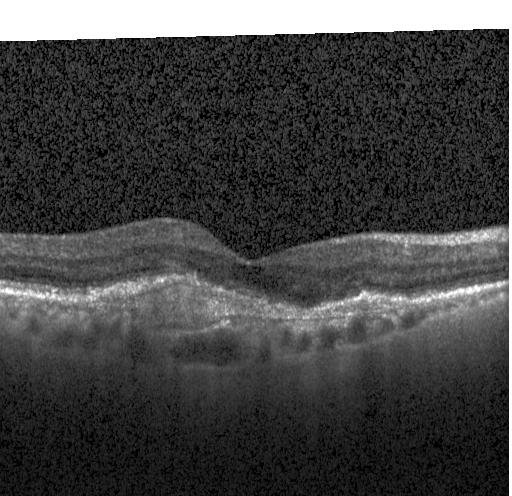 OCT line scan
Impression: CNV.